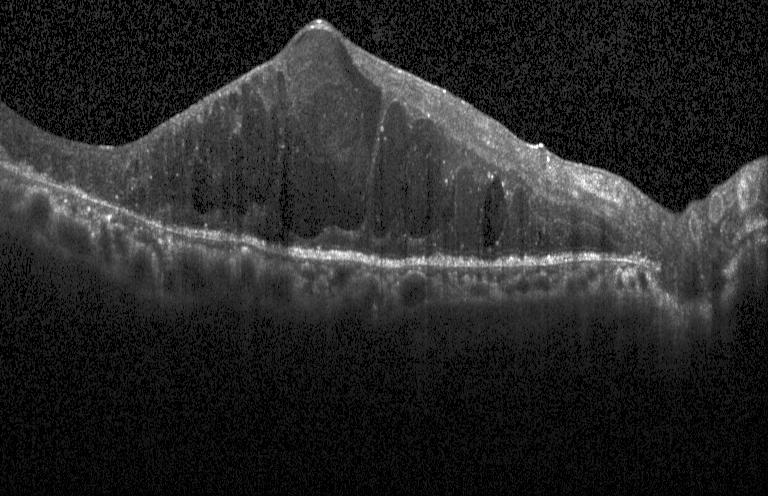

Retinal OCT cross-section, spectral-domain OCT
Diabetic macular edema.